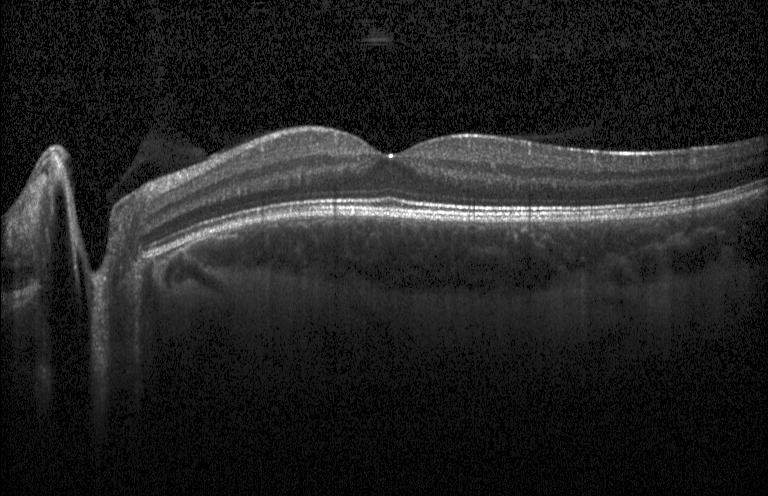 OCT scan showing neither CNV, DME, nor drusen.